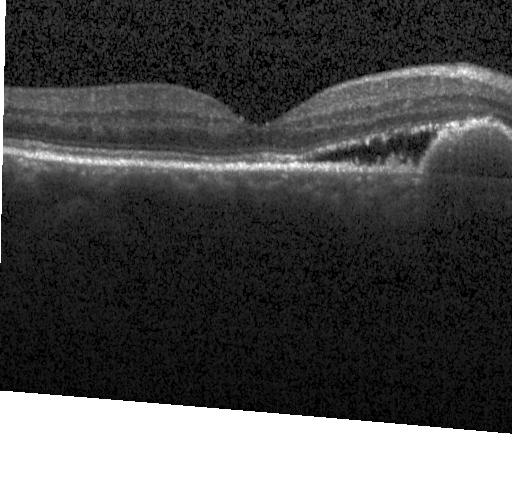

Retinal OCT cross-section showing a choroidal neovascular membrane.